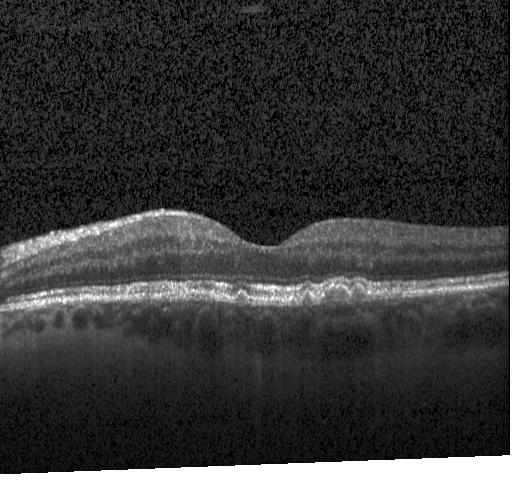 Spectral-domain optical coherence tomography. Optical coherence tomography B-scan — Finding: drusen.